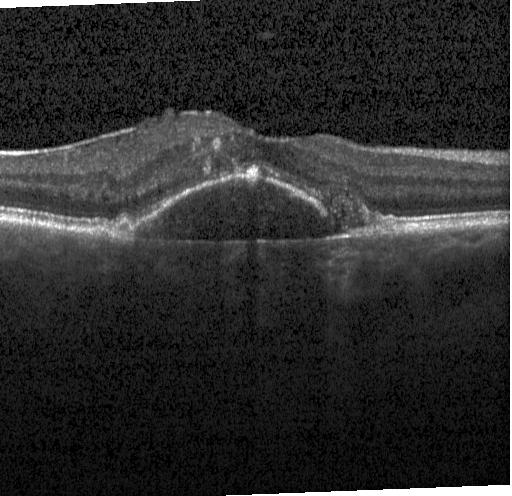
Heidelberg Spectralis OCT system; spectral-domain OCT; OCT line scan.
OCT finding: choroidal neovascularization.